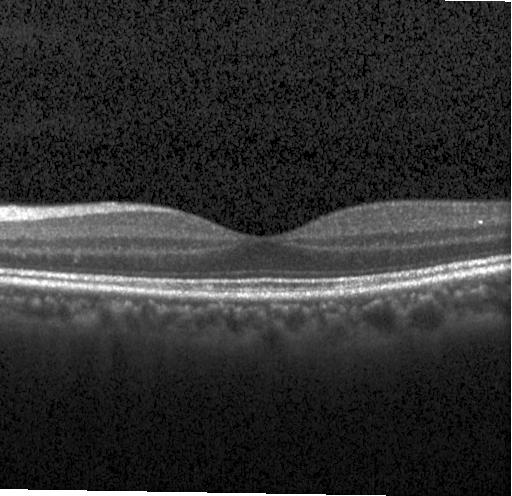 Macular scan; OCT B-scan — OCT finding: no evidence of choroidal neovascularization, diabetic macular edema, or drusen.